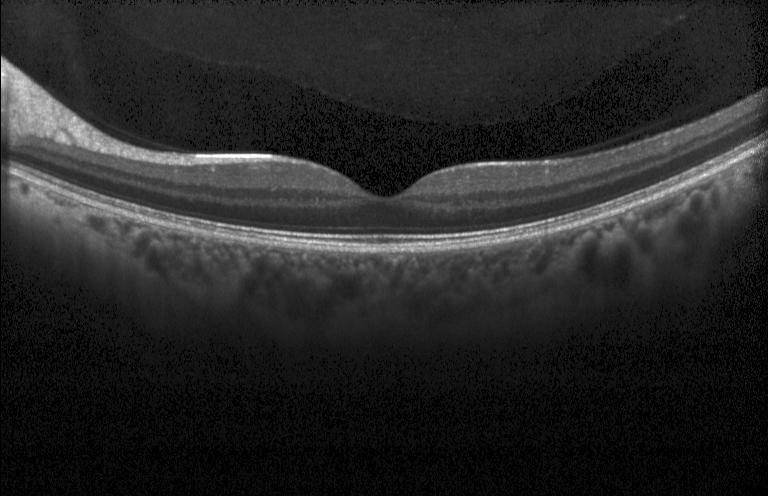

Optical coherence tomography scan, instrument: Heidelberg Spectralis, fovea-centered.
OCT finding: neither choroidal neovascularization, diabetic macular edema, nor drusen.